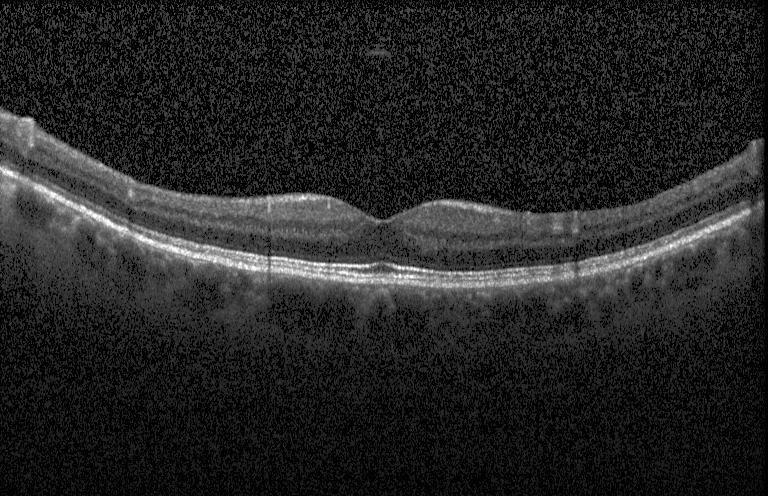

Spectral-domain OCT. Acquired on a Heidelberg Spectralis. Centered on the fovea. Optical coherence tomography B-scan. Dx: no choroidal neovascularization, diabetic macular edema, or drusen.